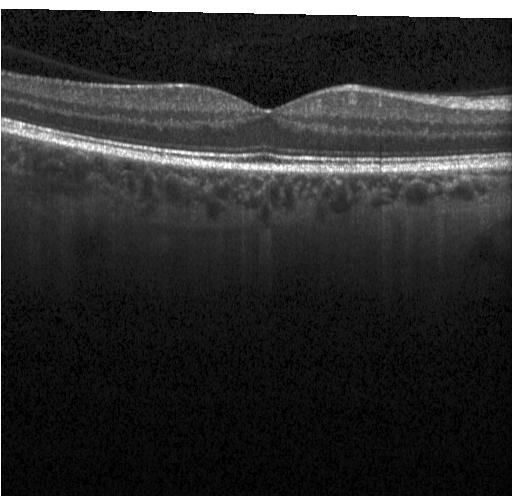 OCT line scan · spectral-domain OCT. Impression: no choroidal neovascularization, no diabetic macular edema, and no drusen.